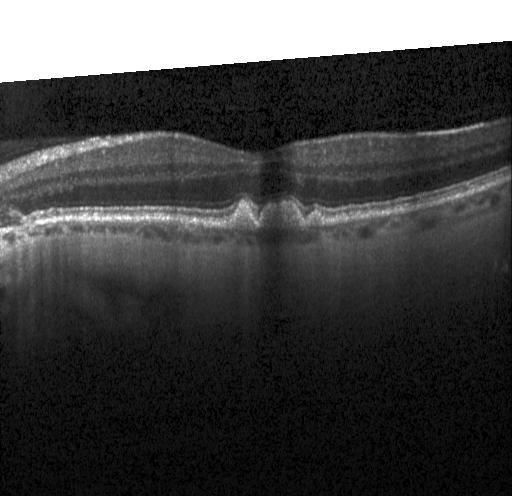

Heidelberg Spectralis OCT system; OCT line scan; horizontal scan through the fovea; SD-OCT.
OCT finding: sub-RPE drusenoid deposits.